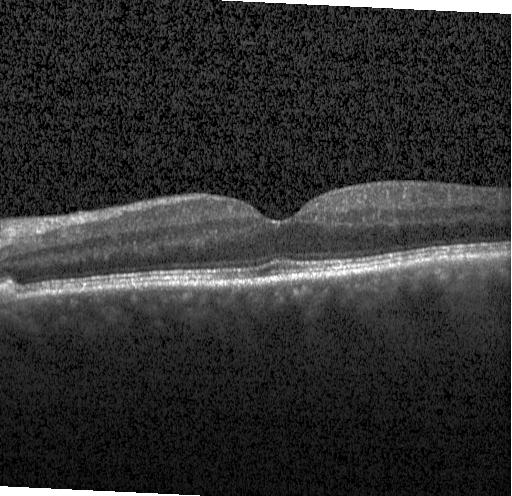

Macular scan · optical coherence tomography B-scan. Finding: no choroidal neovascularization, no diabetic macular edema, and no drusen.